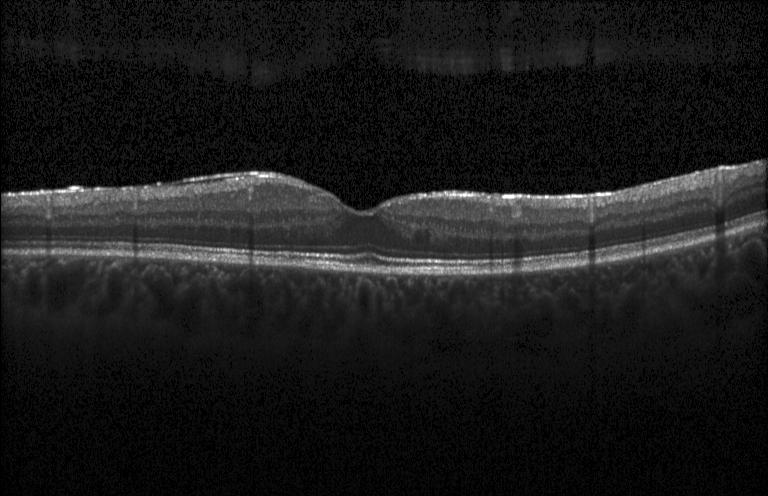
SD-OCT · acquired on a Heidelberg Spectralis · centered on the fovea · retinal OCT cross-section — Dx: no choroidal neovascularization, no diabetic macular edema, and no drusen.